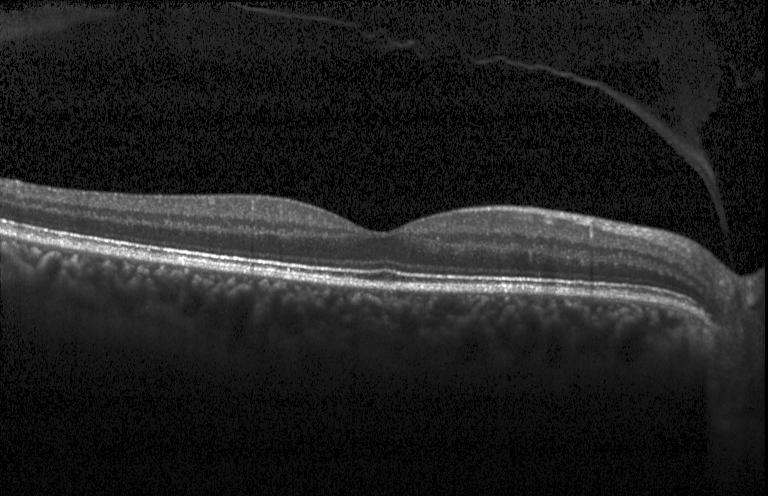

Acquired on a Heidelberg Spectralis. Optical coherence tomography B-scan. Spectral-domain OCT.
Diagnosis: no choroidal neovascularization, no diabetic macular edema, and no drusen.